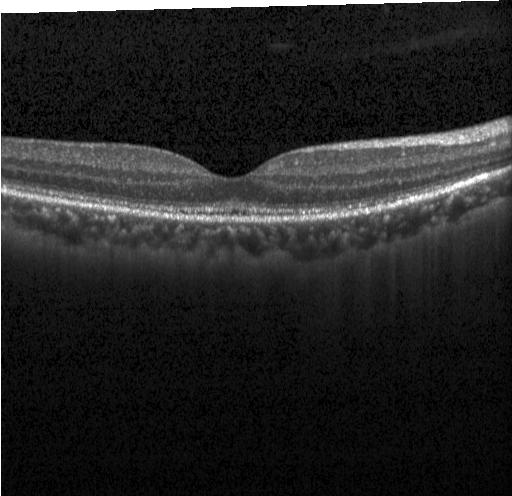

Diagnosis: no CNV, DME, or drusen.